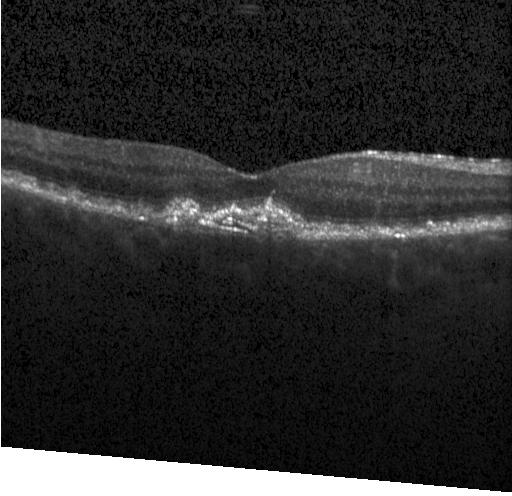

Macular scan; retinal OCT B-scan; Heidelberg Spectralis; spectral-domain OCT — Assessment: CNV.